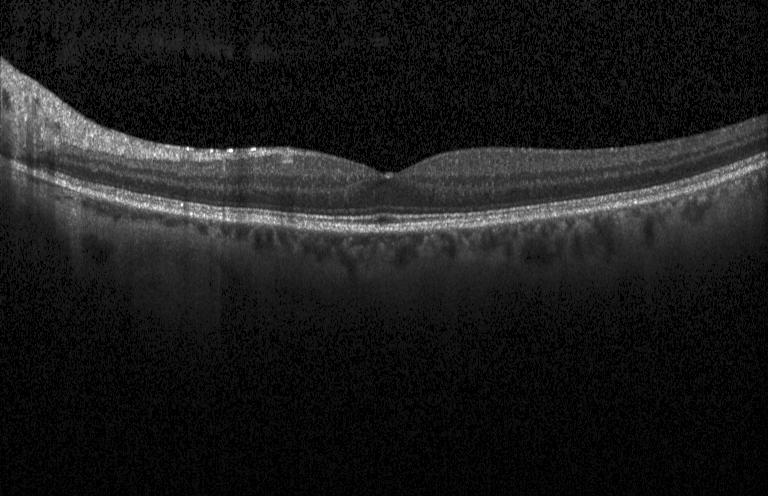 The scan shows neither CNV, DME, nor drusen.